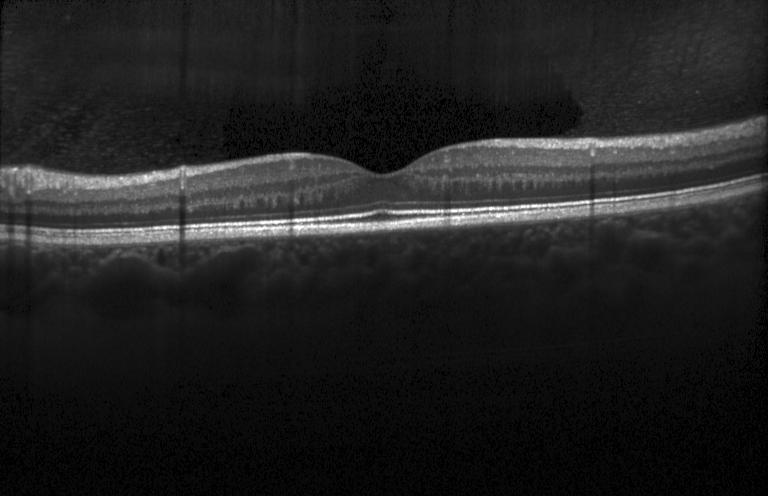

Retinal OCT B-scan — This B-scan demonstrates no evidence of choroidal neovascularization, diabetic macular edema, or drusen.